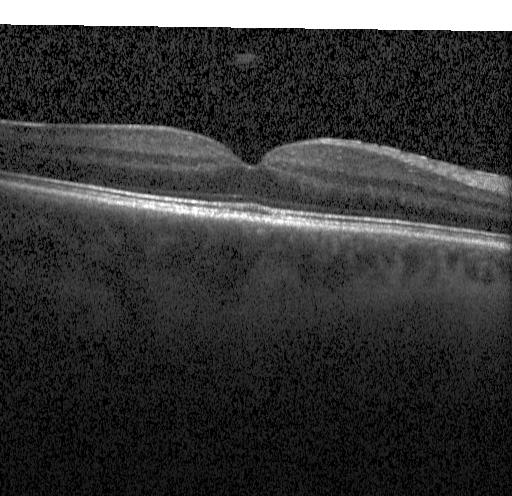
Optical coherence tomography scan.
The scan shows no CNV, no DME, and no drusen.